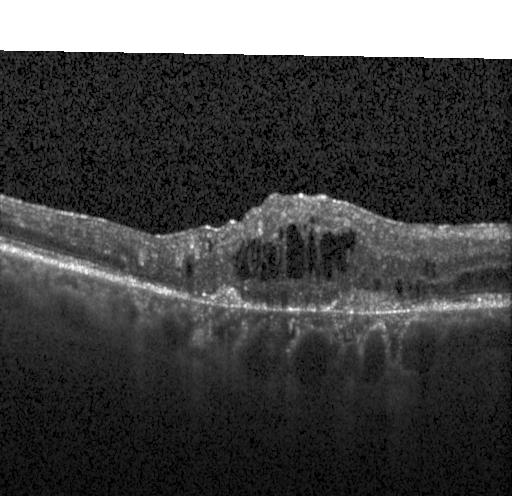

SD-OCT; retinal OCT B-scan
A choroidal neovascular membrane.